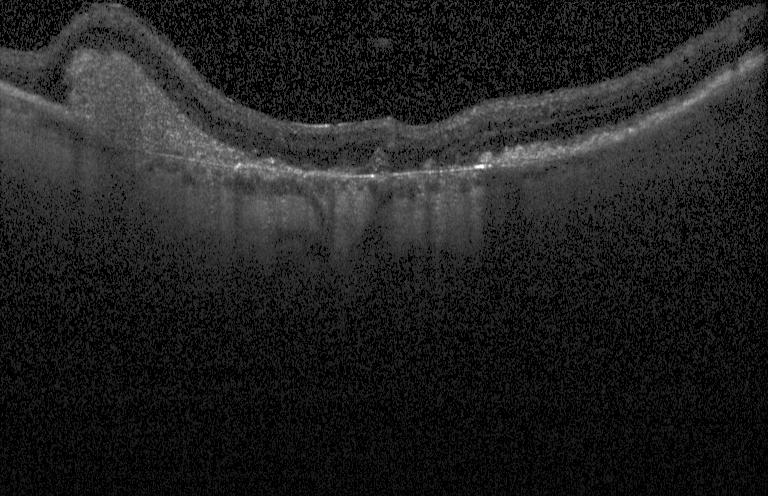

Optical coherence tomography B-scan; through the macula; Heidelberg Spectralis OCT system — Impression: CNV.